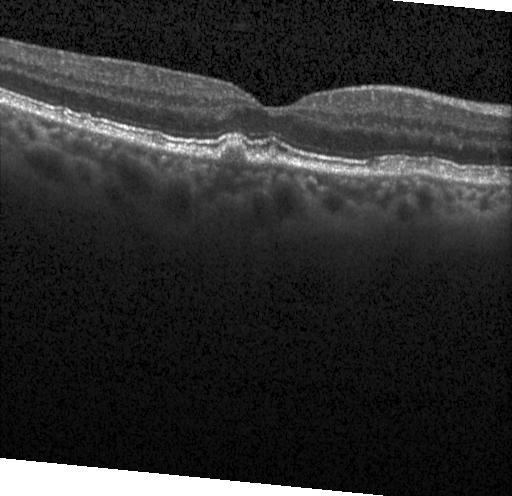 Acquired on a Heidelberg Spectralis; spectral-domain OCT; optical coherence tomography B-scan
Finding: drusen.